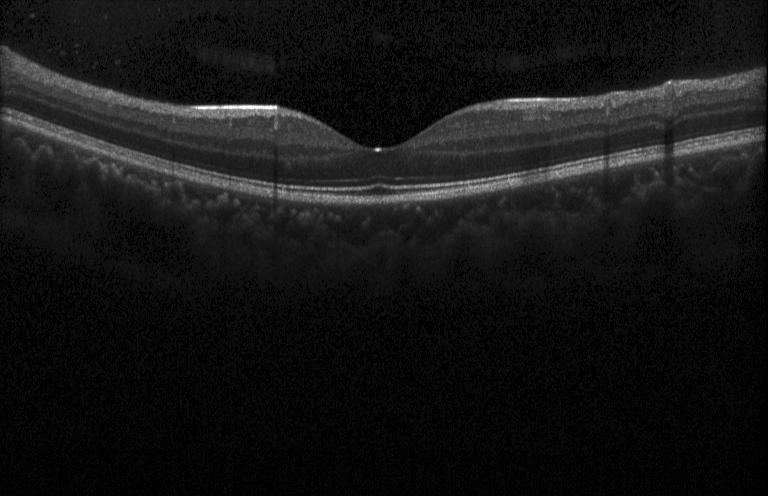

Retinal OCT cross-section — Diagnosis: no choroidal neovascularization, no diabetic macular edema, and no drusen.